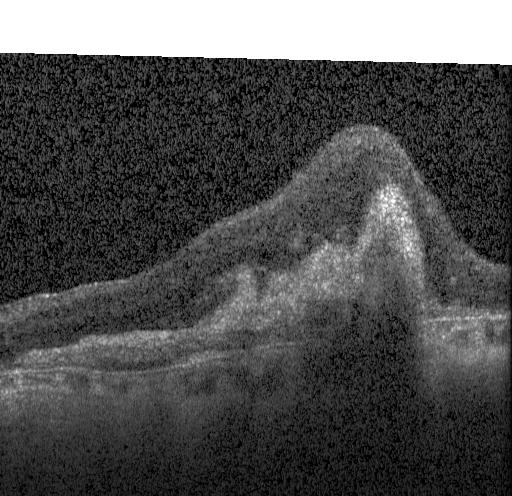 CNV.